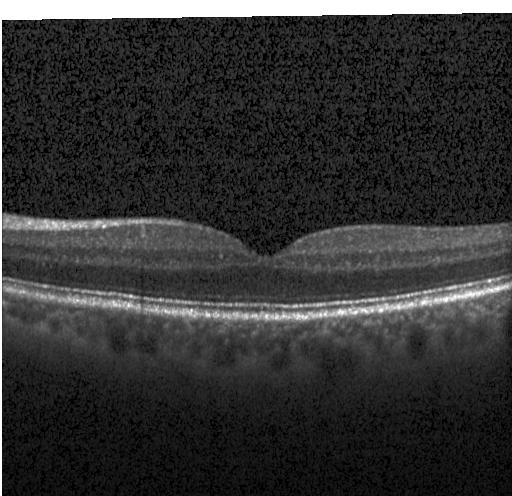 Retinal OCT B-scan. Finding: neither choroidal neovascularization, diabetic macular edema, nor drusen.